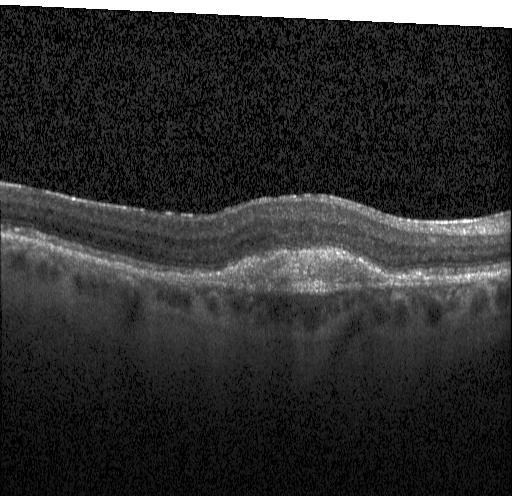

Spectral-domain optical coherence tomography · OCT B-scan · through the macula · Heidelberg Spectralis — Finding: a choroidal neovascular membrane.